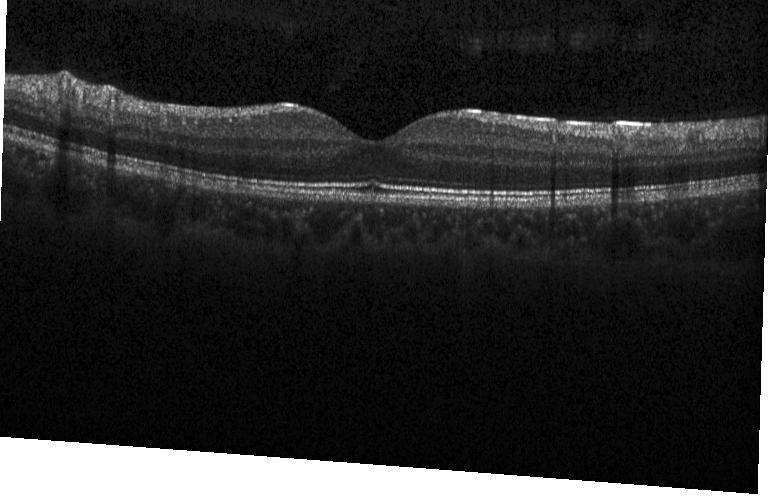
Optical coherence tomography scan
Diagnosis: no CNV, no DME, and no drusen.